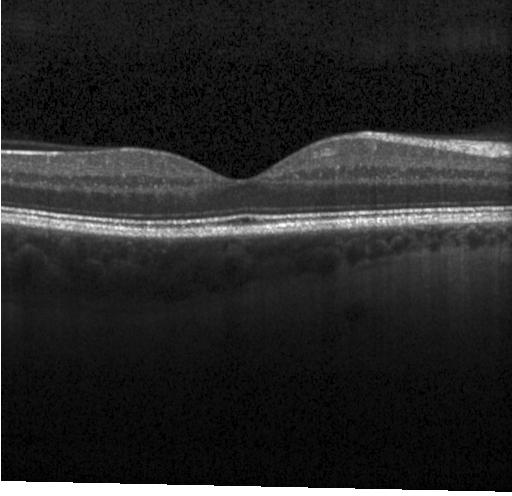 Through the macula; SD-OCT; Heidelberg Spectralis OCT system; OCT B-scan. The scan shows no evidence of choroidal neovascularization, diabetic macular edema, or drusen.